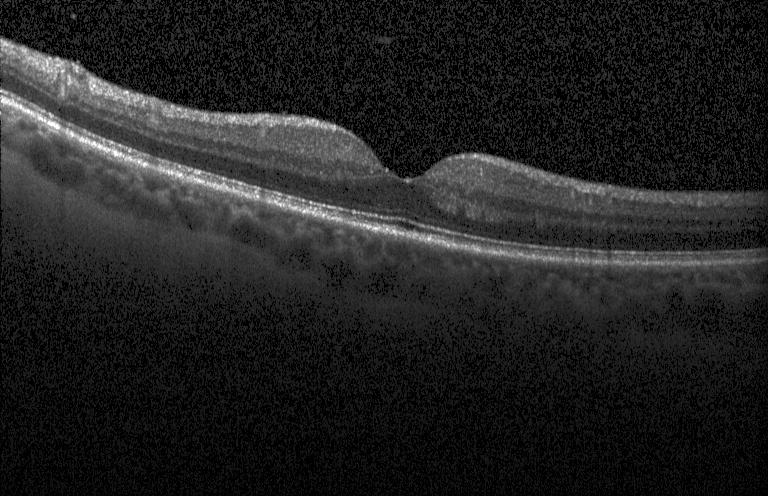

Spectral-domain OCT B-scan: neither CNV, DME, nor drusen.